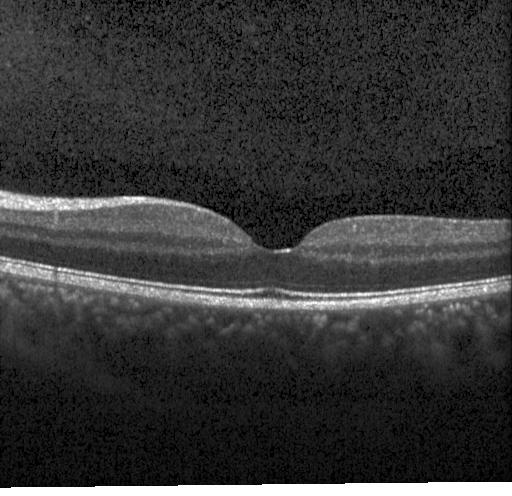
Spectral-domain OCT, OCT B-scan
Macular OCT: no CNV, no DME, and no drusen.